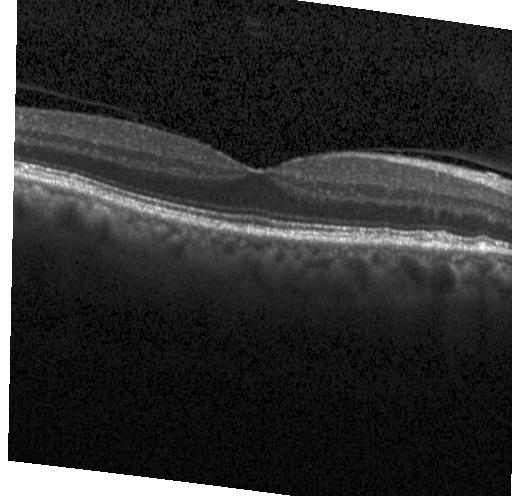 Through the macula. Acquired on a Heidelberg Spectralis. Optical coherence tomography scan — Impression: drusen.